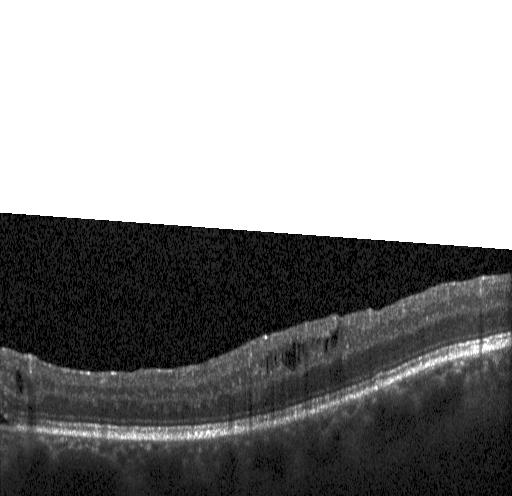 Instrument: Heidelberg Spectralis. SD-OCT. Optical coherence tomography scan
Finding: diabetic macular edema.